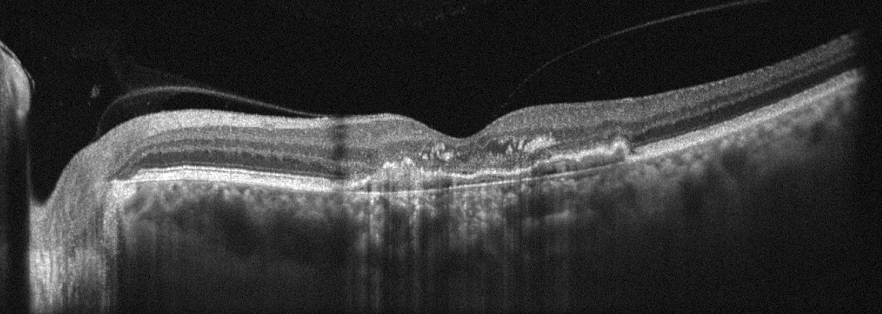
Left eye; optical coherence tomography scan — Diagnosis: age-related macular degeneration (AMD).